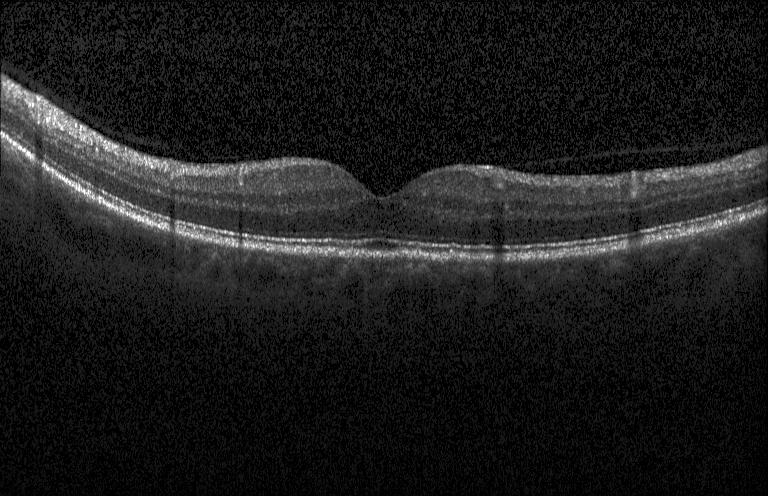 OCT line scan. Horizontal scan through the fovea. Acquired on a Heidelberg Spectralis — Diagnosis: no choroidal neovascularization, diabetic macular edema, or drusen.